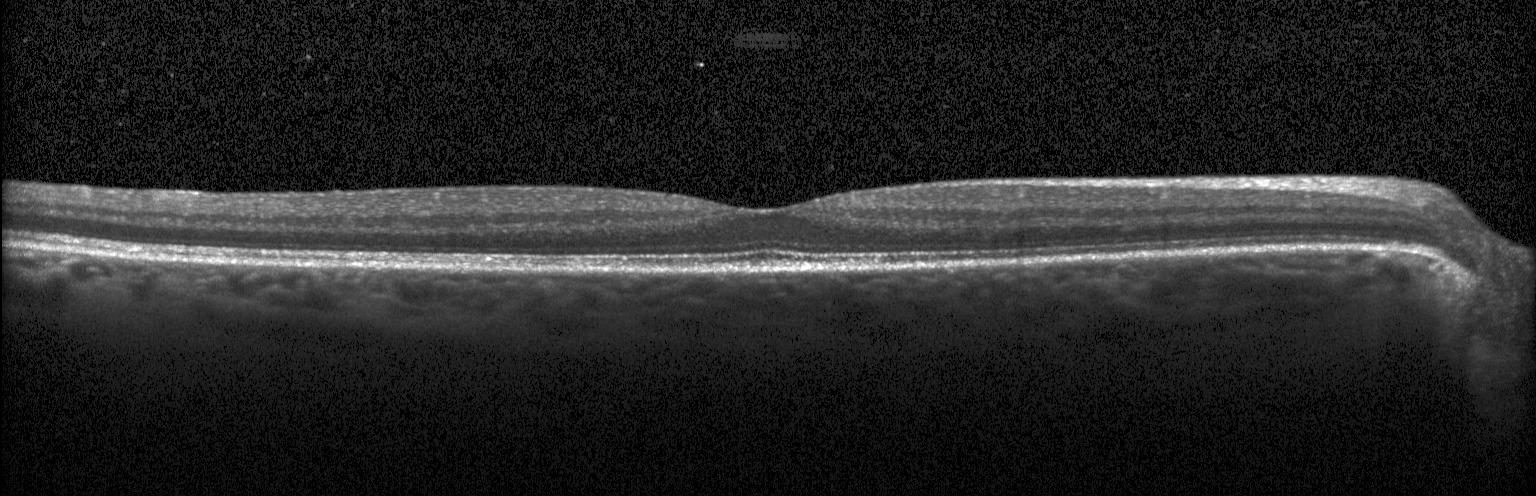
Heidelberg Spectralis · optical coherence tomography B-scan — No CNV, no DME, and no drusen.